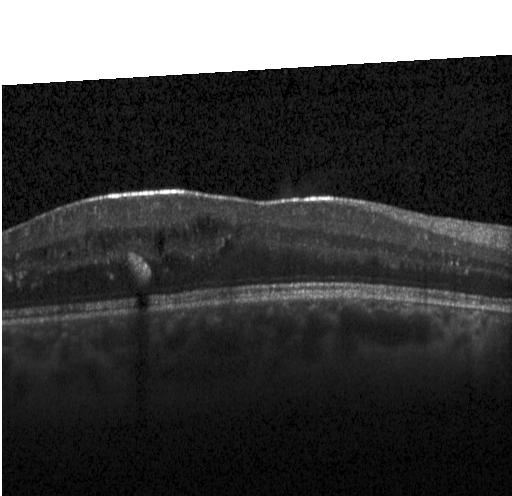

Dx: DME.